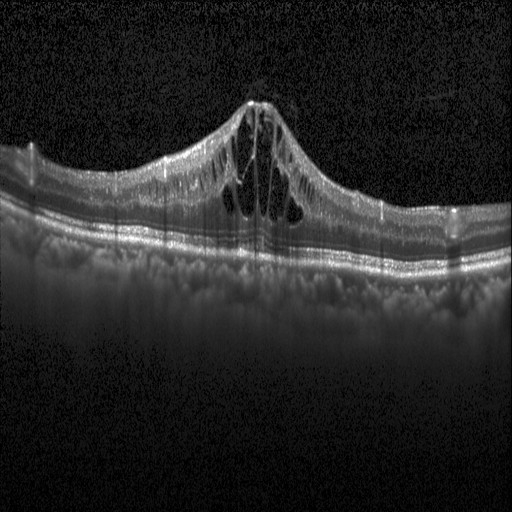

OCT B-scan. The scan shows diabetic macular edema.